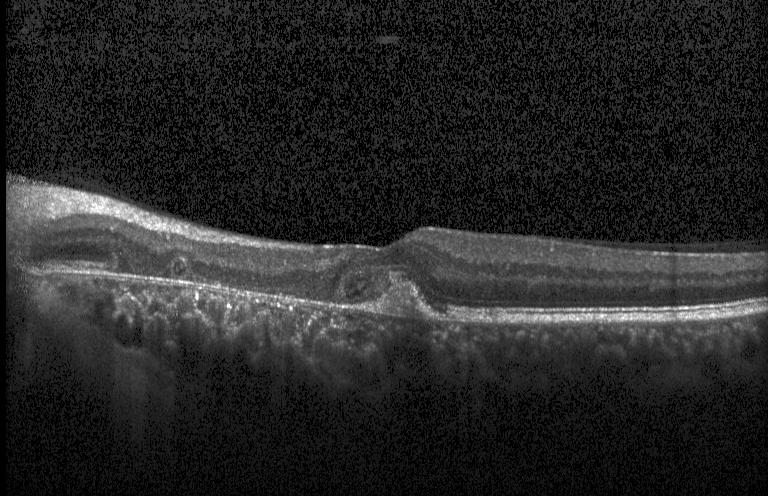

Spectral-domain OCT B-scan: CNV.